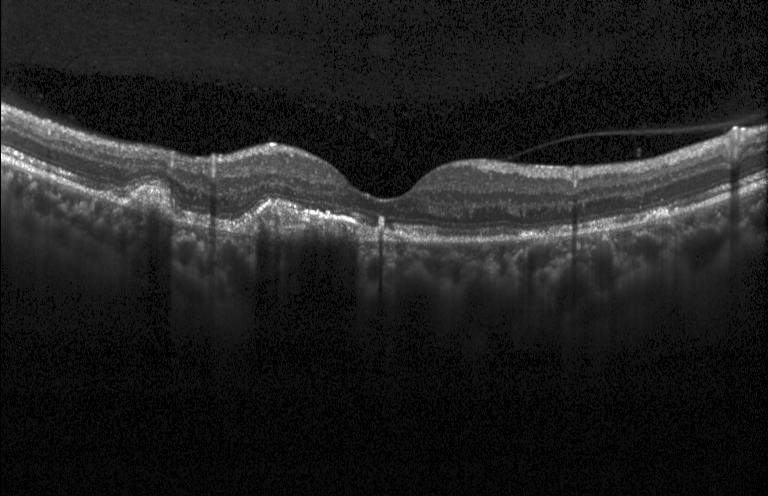

This B-scan demonstrates a choroidal neovascular membrane.